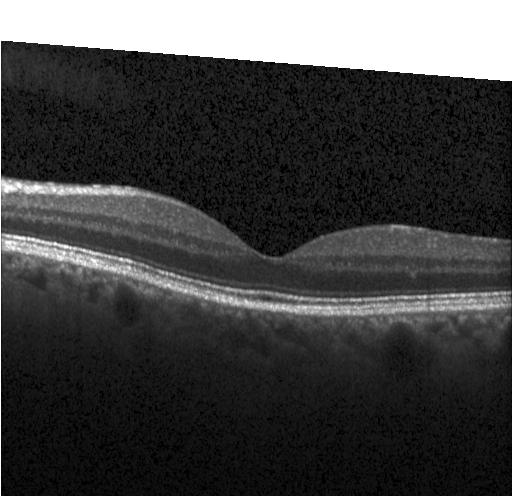

Macular OCT: no choroidal neovascularization, no diabetic macular edema, and no drusen.